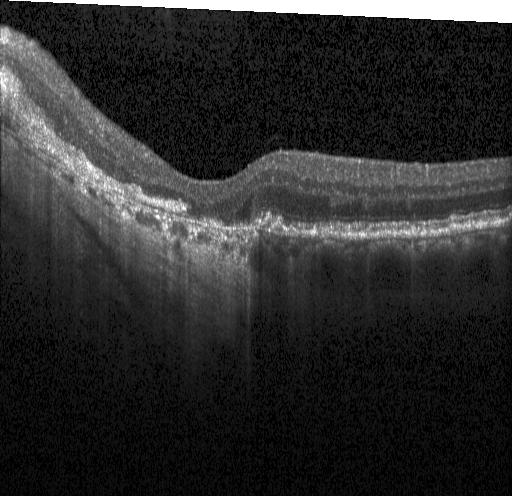

Macular OCT demonstrating a choroidal neovascular membrane.